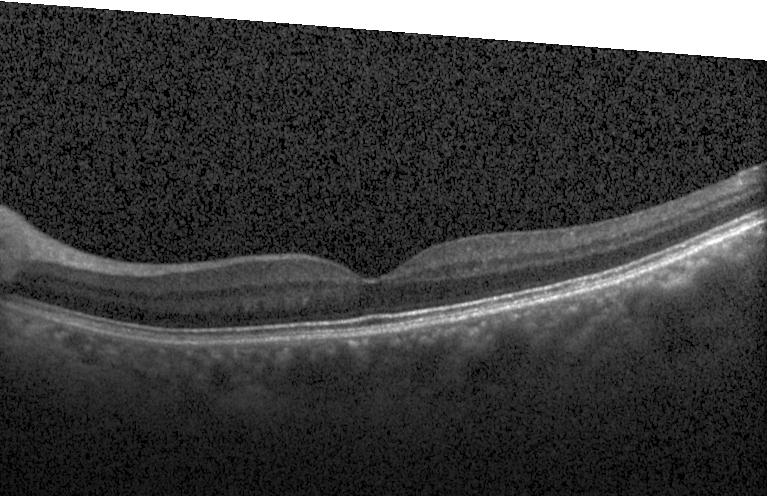 Heidelberg Spectralis OCT system, spectral-domain optical coherence tomography, retinal OCT cross-section, horizontal scan through the fovea. Macular OCT: no choroidal neovascularization, no diabetic macular edema, and no drusen.